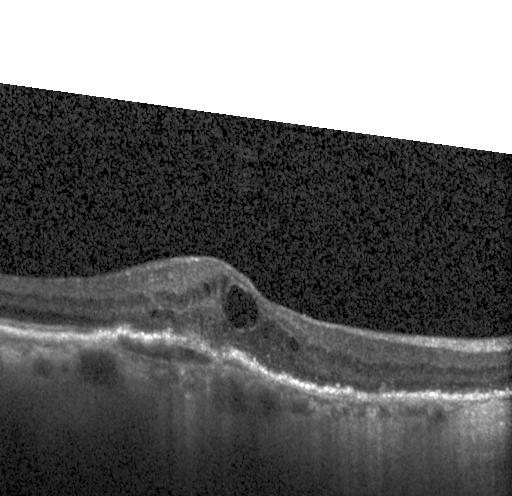 Retinal OCT B-scan
The scan shows choroidal neovascularization (CNV).